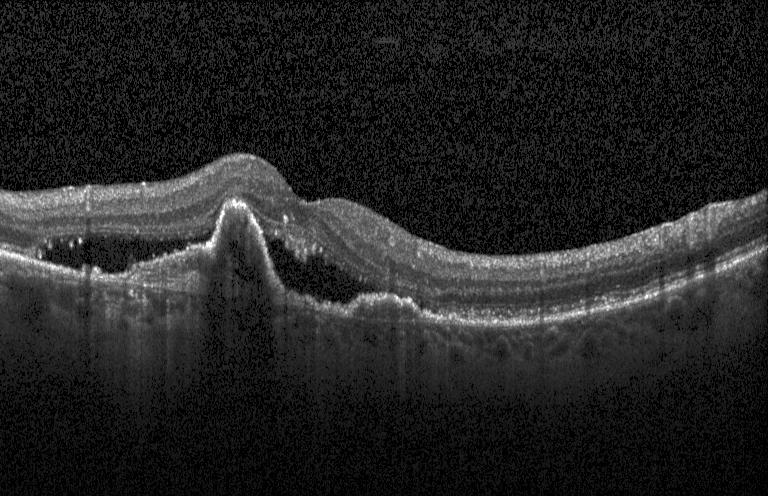

OCT finding: choroidal neovascularization.